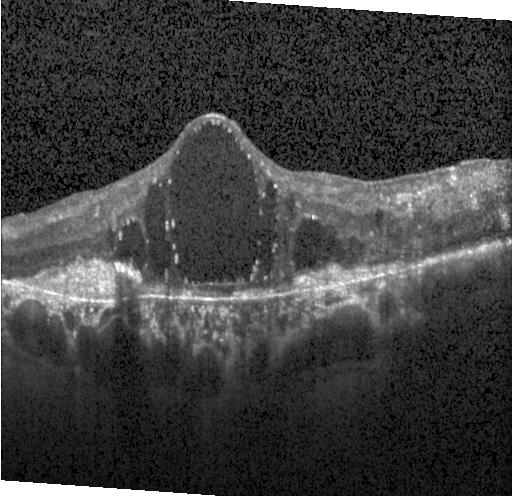 Optical coherence tomography B-scan; Heidelberg Spectralis.
Finding: a choroidal neovascular membrane.